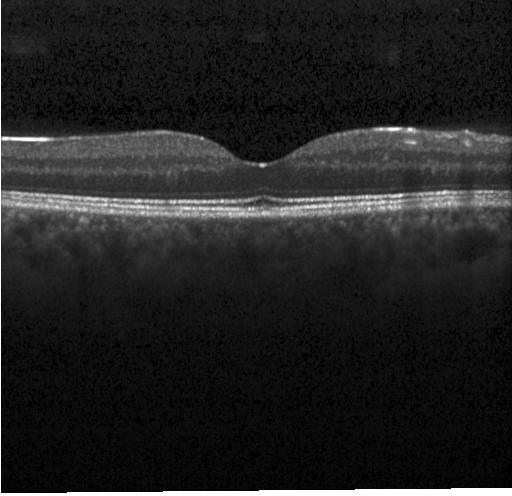

OCT scan showing no evidence of choroidal neovascularization, diabetic macular edema, or drusen.